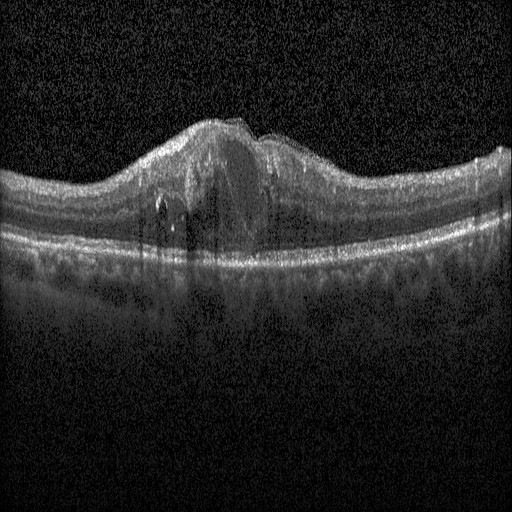
Spectral-domain OCT · Heidelberg Spectralis · OCT line scan · centered on the fovea. Dx: diabetic macular edema.